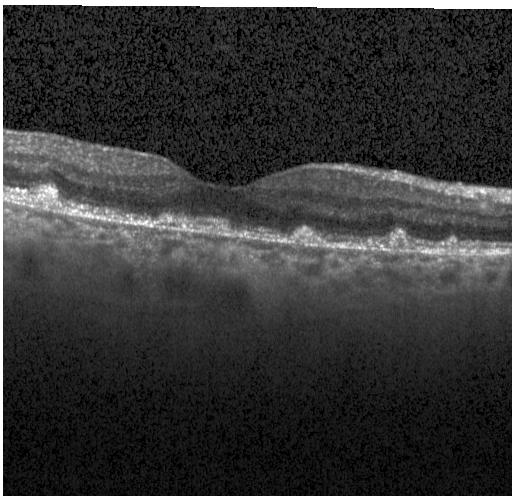

Diagnosis: choroidal neovascularization (CNV).